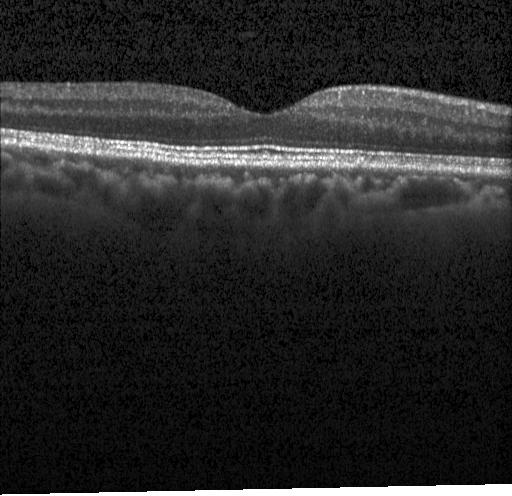 Spectral-domain OCT B-scan: no choroidal neovascularization, diabetic macular edema, or drusen.